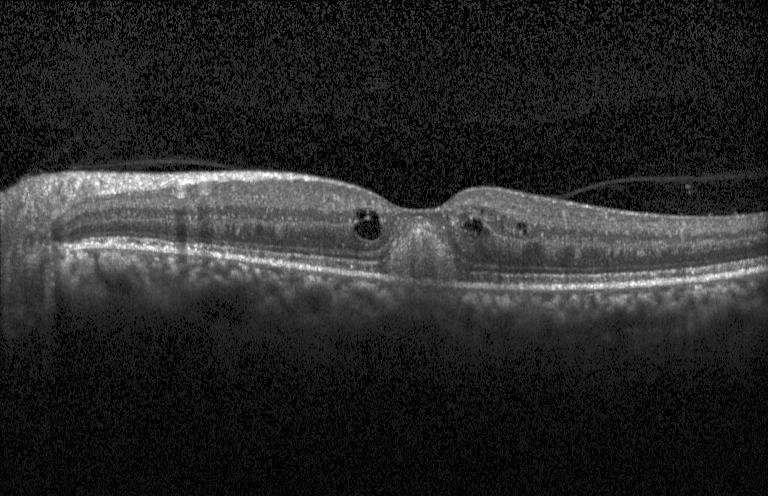

Impression: choroidal neovascularization.